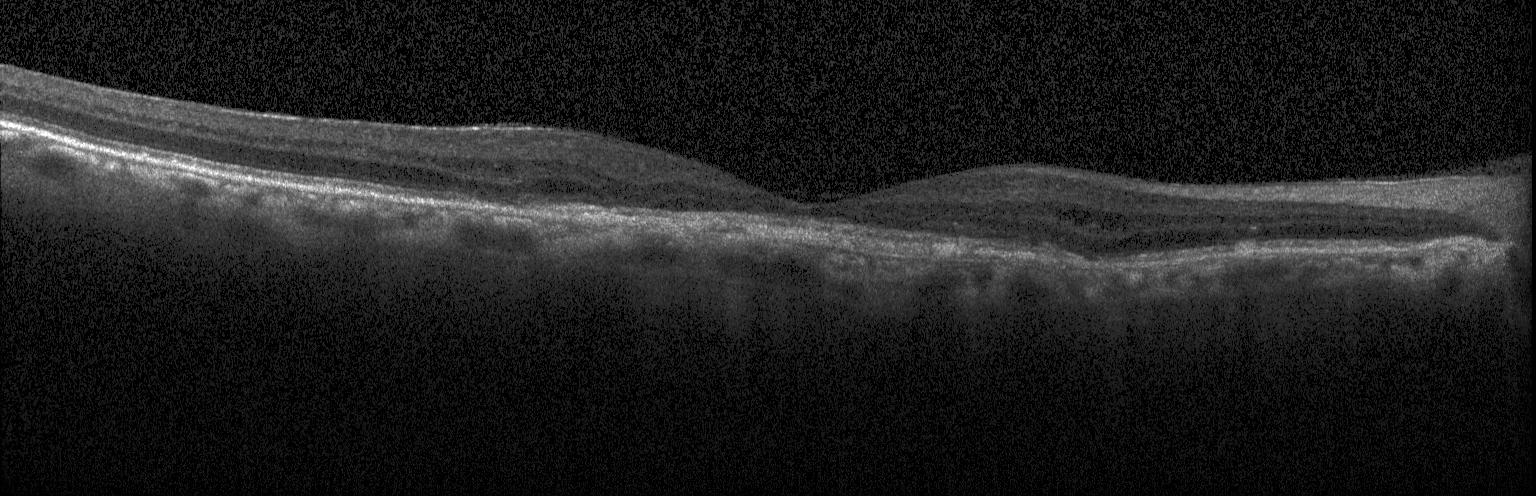 Optical coherence tomography scan. Through the macula. Acquired on a Heidelberg Spectralis. Spectral-domain optical coherence tomography
Assessment: choroidal neovascularization (CNV).